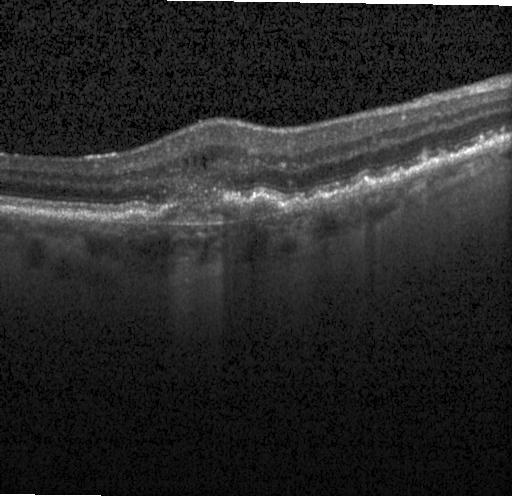 Diagnosis: choroidal neovascularization.